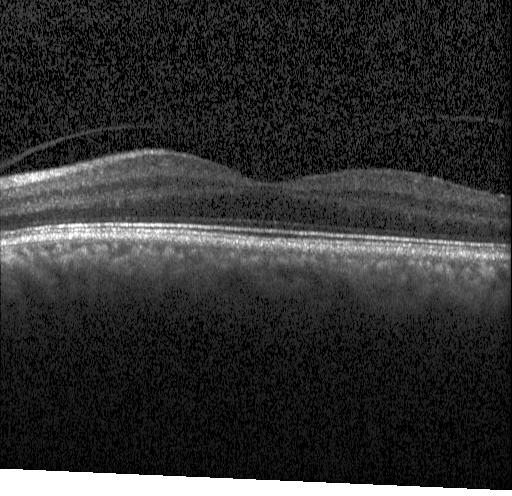
Dx: neither CNV, DME, nor drusen.